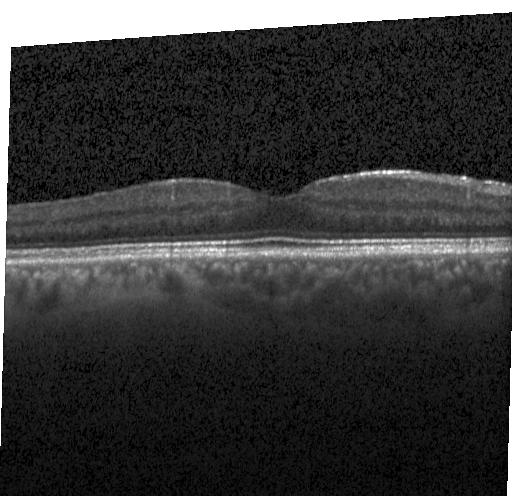
Retinal OCT B-scan, instrument: Heidelberg Spectralis
Assessment: no CNV, DME, or drusen.